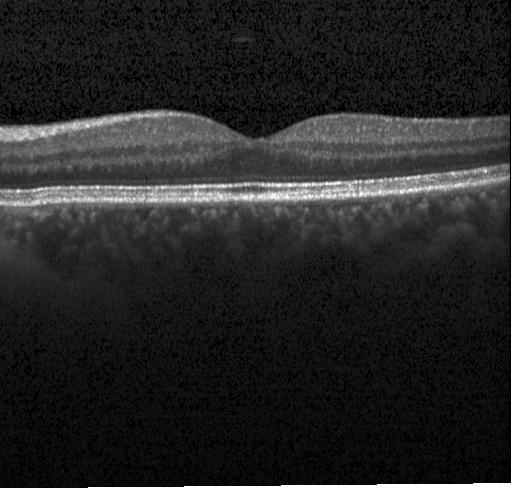 Spectral-domain optical coherence tomography. Centered on the fovea. Optical coherence tomography scan. The scan shows no CNV, DME, or drusen.